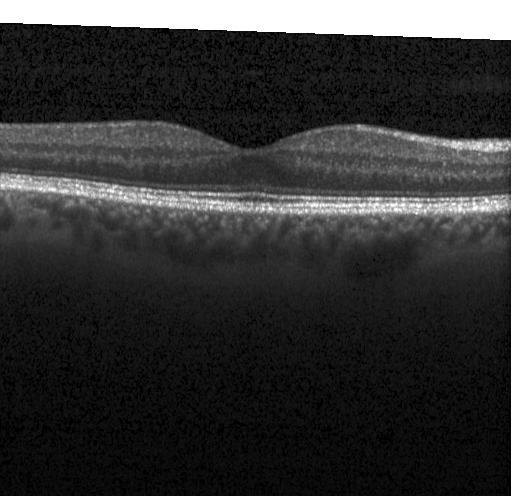 OCT B-scan, SD-OCT, centered on the fovea — This B-scan demonstrates neither CNV, DME, nor drusen.